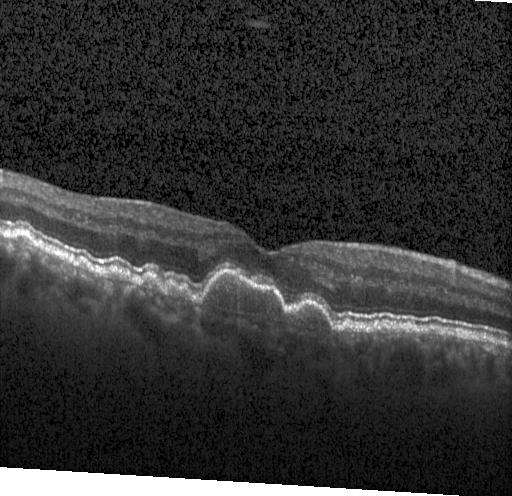
Spectral-domain optical coherence tomography; optical coherence tomography B-scan
This B-scan demonstrates multiple drusen.